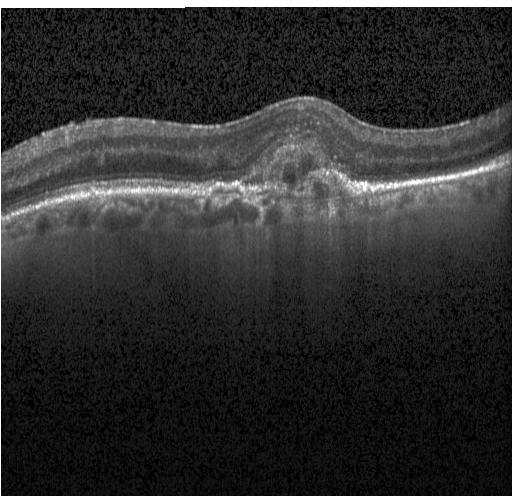

OCT B-scan. Macular OCT: choroidal neovascularization.